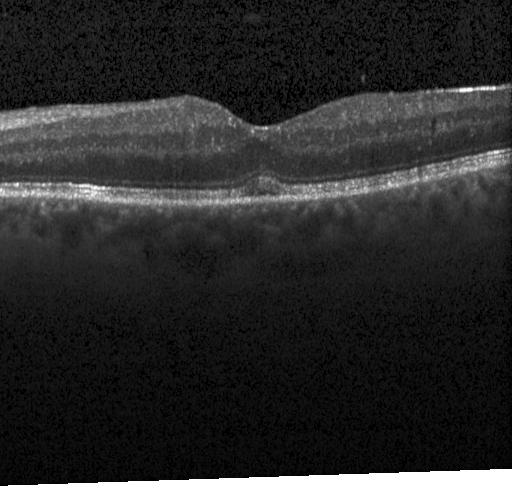 Spectral-domain optical coherence tomography; macular scan; OCT line scan; instrument: Heidelberg Spectralis.
This B-scan demonstrates DME.